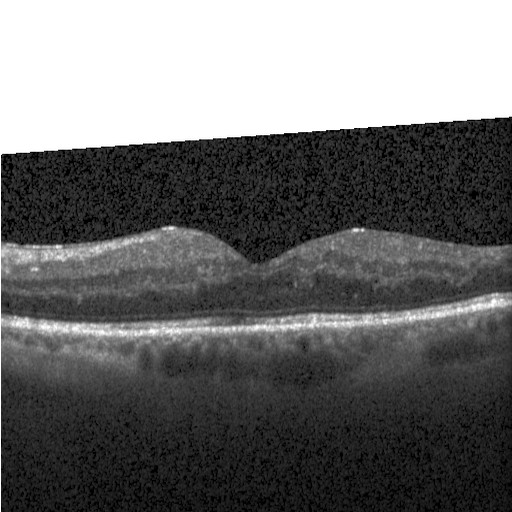

This B-scan demonstrates diabetic macular edema (DME).